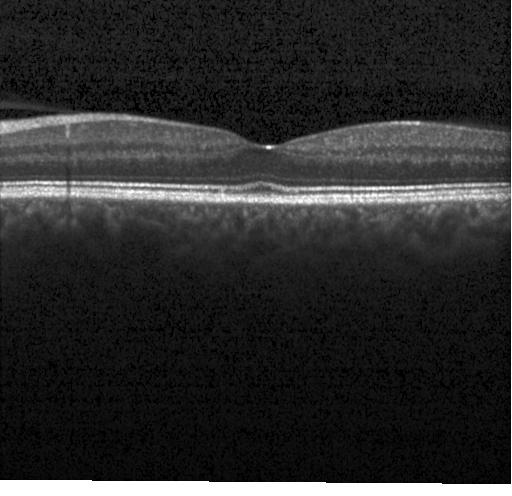

Spectral-domain OCT B-scan: neither CNV, DME, nor drusen.